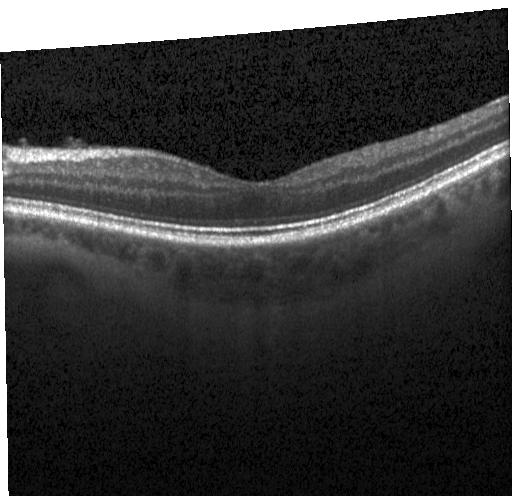 Optical coherence tomography B-scan
This B-scan demonstrates neither CNV, DME, nor drusen.